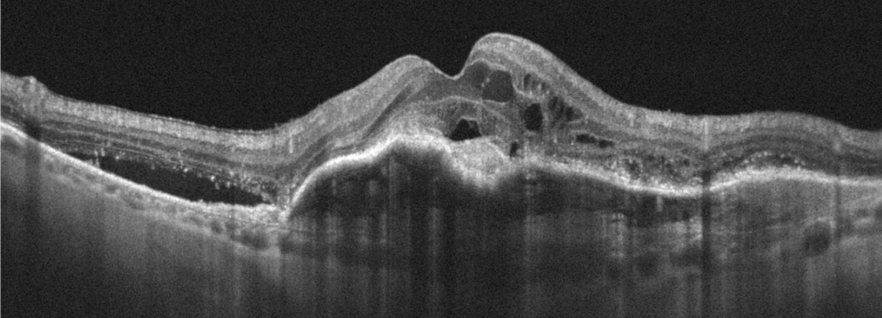 OCT line scan
This B-scan demonstrates age-related macular degeneration.